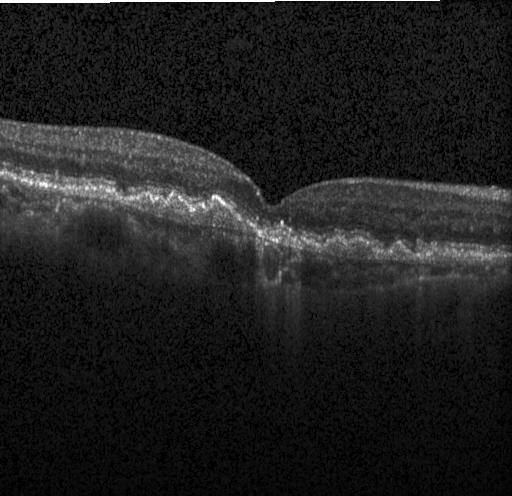

Centered on the fovea; SD-OCT; optical coherence tomography B-scan; acquired on a Heidelberg Spectralis. Finding: a choroidal neovascular membrane.